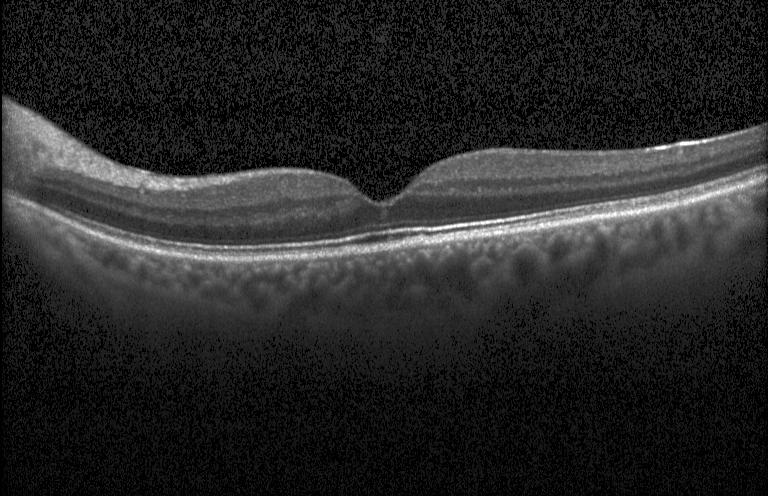
Instrument: Heidelberg Spectralis. SD-OCT. OCT B-scan — Finding: no evidence of choroidal neovascularization, diabetic macular edema, or drusen.